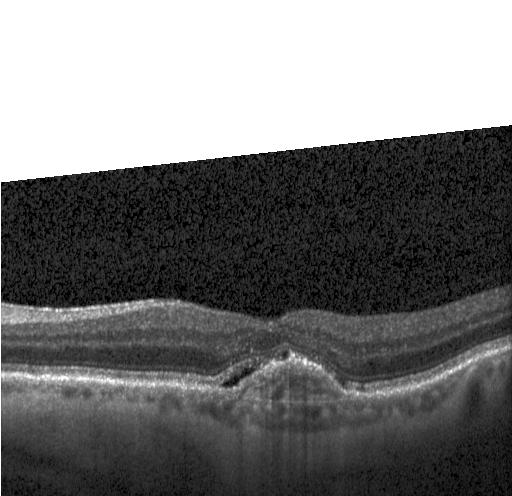

Optical coherence tomography B-scan
Diagnosis: CNV.